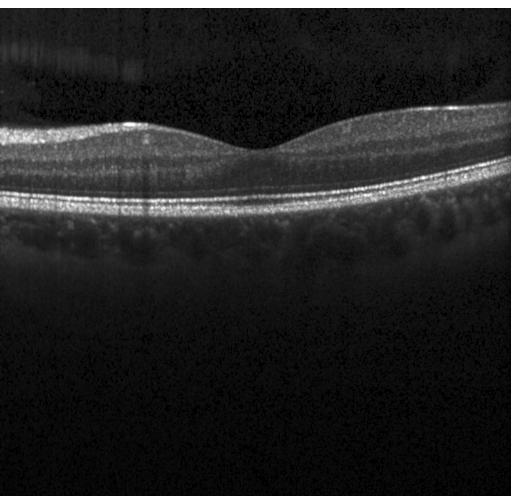 Retinal OCT cross-section. Fovea-centered
Neither choroidal neovascularization, diabetic macular edema, nor drusen.